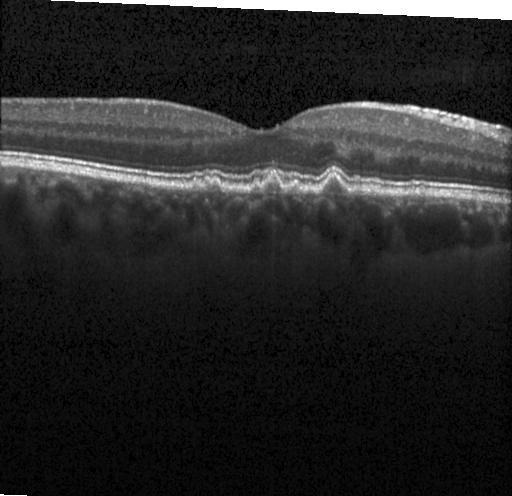
OCT B-scan
This B-scan demonstrates multiple drusen.